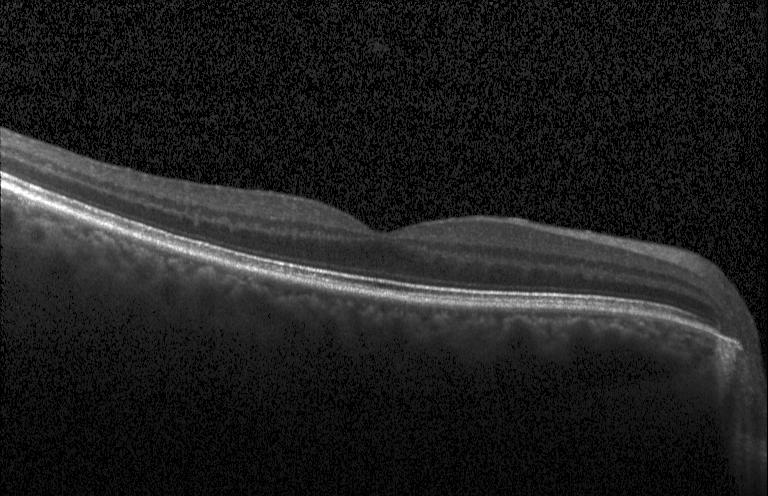
Spectral-domain optical coherence tomography, centered on the fovea, retinal OCT cross-section. OCT finding: no evidence of CNV, DME, or drusen.